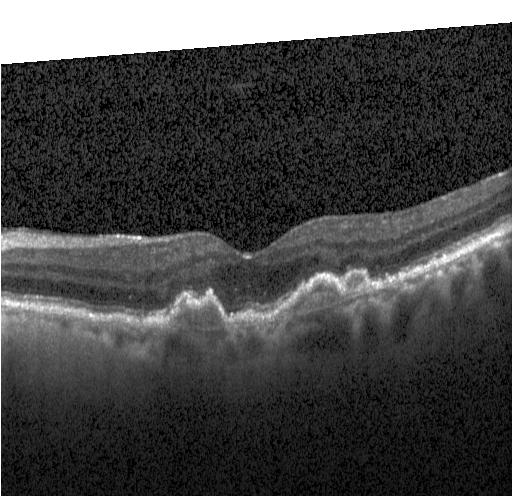
Diagnosis: CNV.